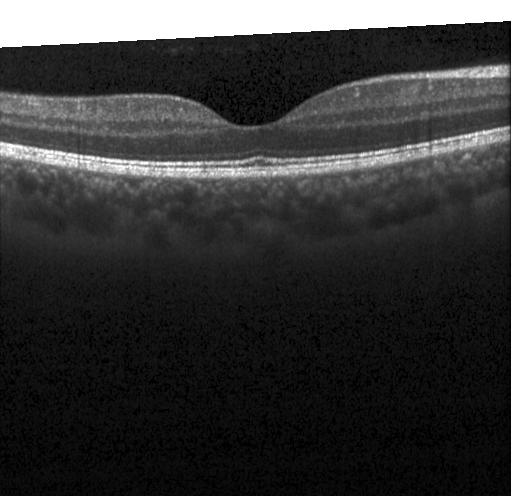
OCT line scan · Heidelberg Spectralis OCT system · spectral-domain OCT · through the macula — The scan shows neither CNV, DME, nor drusen.